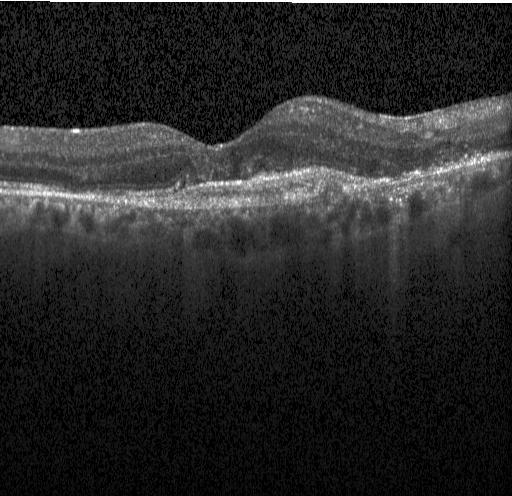

Spectral-domain optical coherence tomography · retinal OCT cross-section · instrument: Heidelberg Spectralis · fovea-centered.
Dx: a choroidal neovascular membrane.